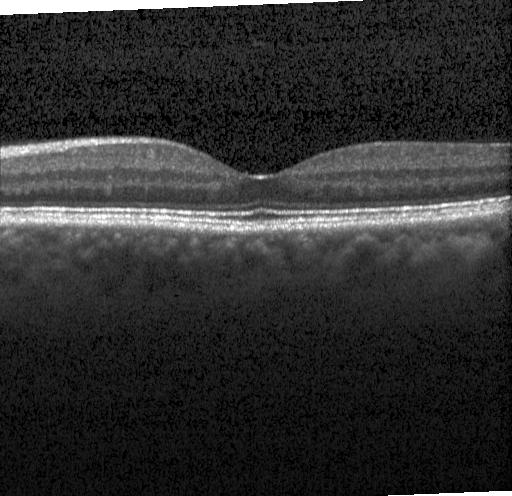 Spectral-domain OCT; instrument: Heidelberg Spectralis; optical coherence tomography scan
No evidence of choroidal neovascularization, diabetic macular edema, or drusen.